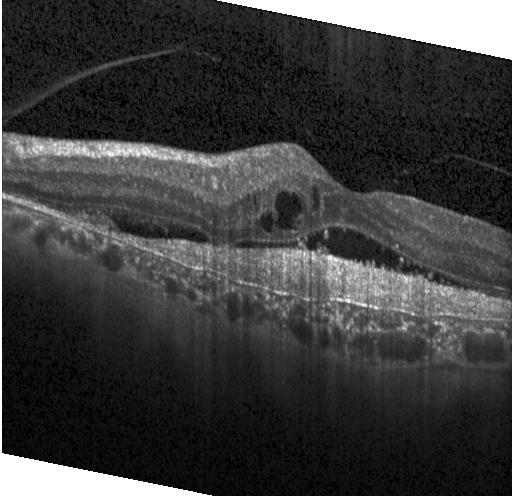
Retinal OCT B-scan.
Dx: CNV.